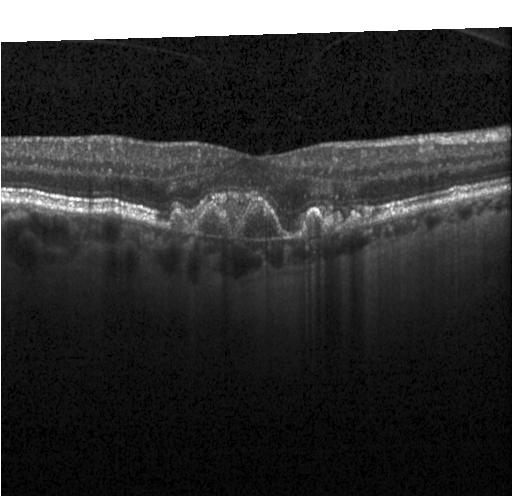

Finding: CNV.